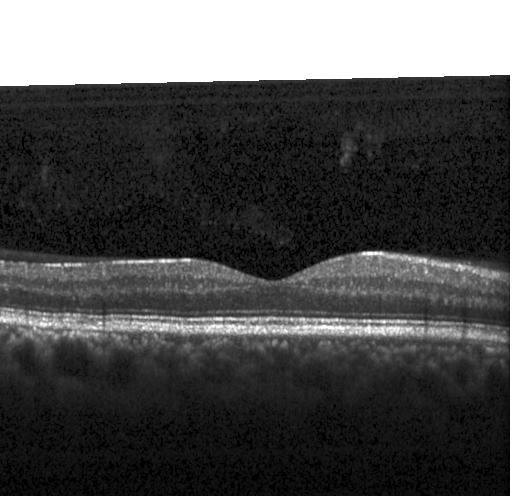
Retinal OCT cross-section.
Impression: no evidence of CNV, DME, or drusen.